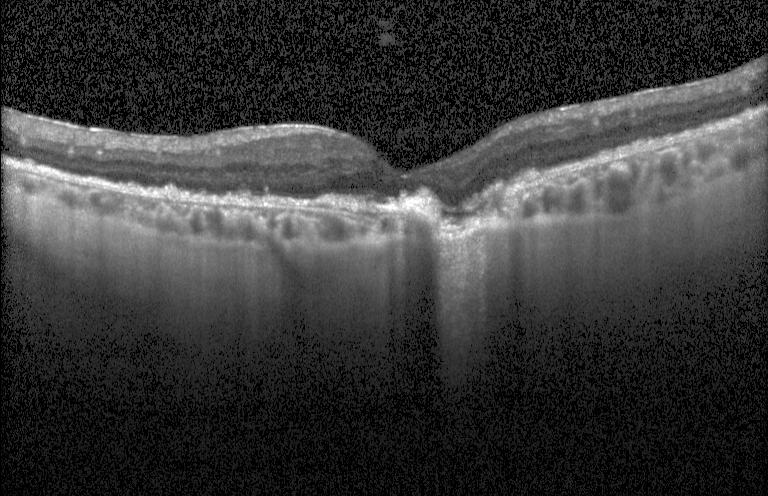
Macular OCT demonstrating a choroidal neovascular membrane.